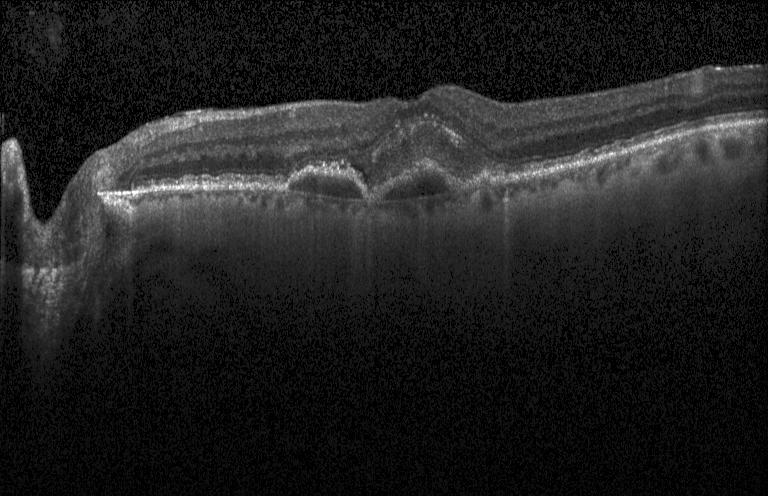

Finding: choroidal neovascularization (CNV).